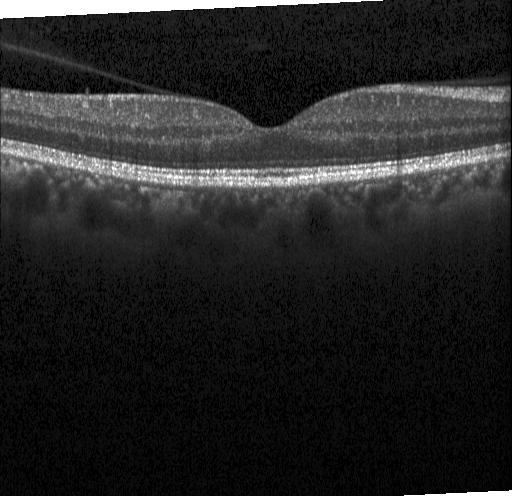 Heidelberg Spectralis OCT system. Optical coherence tomography B-scan. Macular scan
No evidence of choroidal neovascularization, diabetic macular edema, or drusen.